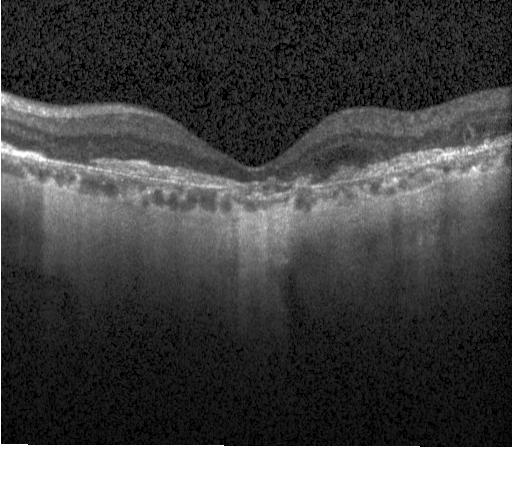
Impression: choroidal neovascularization.